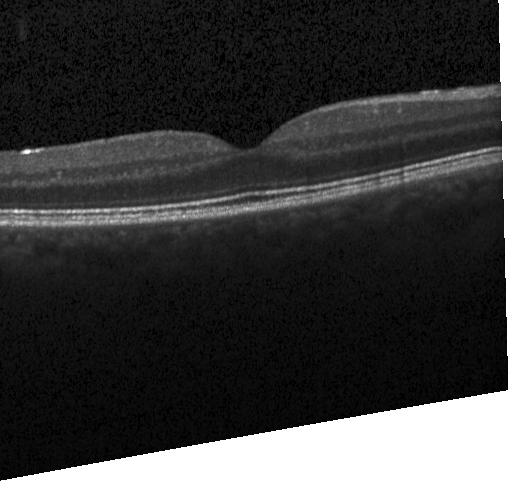

Assessment: neither choroidal neovascularization, diabetic macular edema, nor drusen.